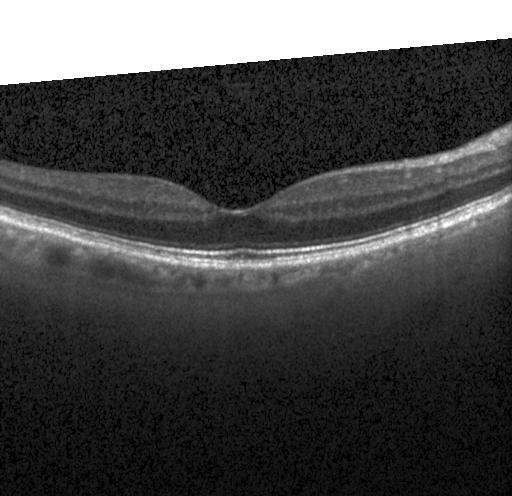 Optical coherence tomography B-scan · Heidelberg Spectralis. Impression: no choroidal neovascularization, no diabetic macular edema, and no drusen.